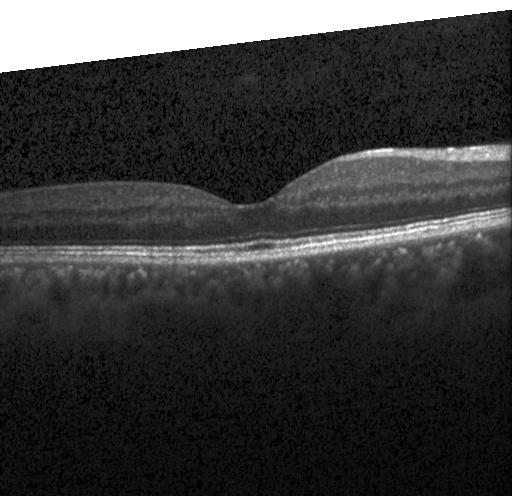
Fovea-centered; SD-OCT; acquired on a Heidelberg Spectralis; OCT line scan
No evidence of choroidal neovascularization, diabetic macular edema, or drusen.